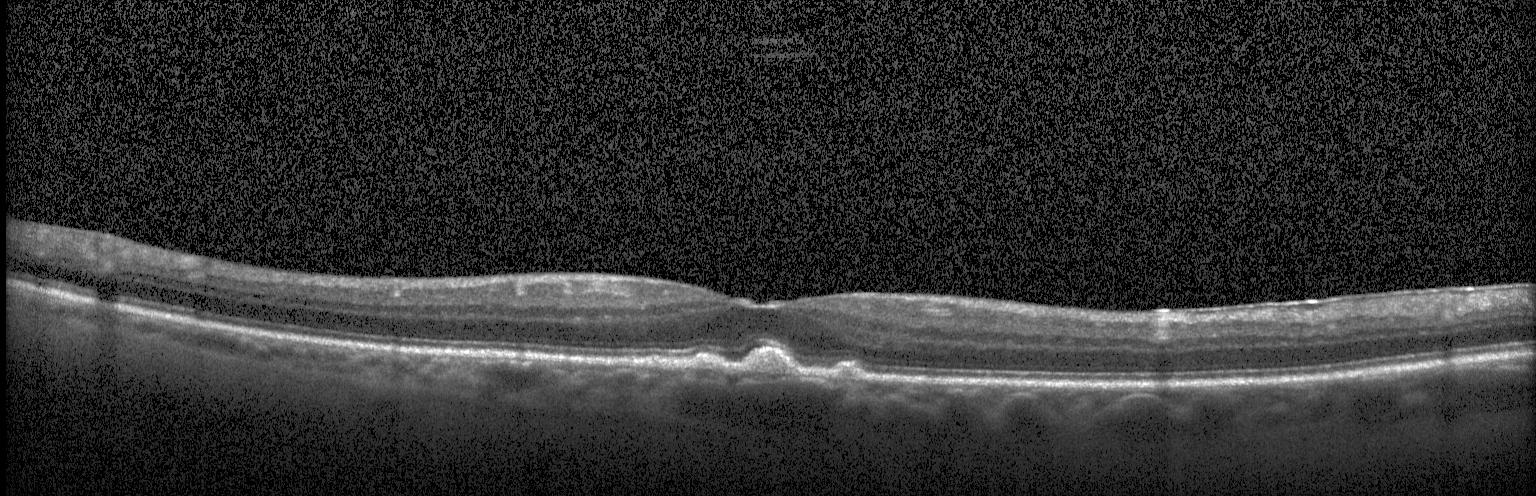
Heidelberg Spectralis OCT system; retinal OCT cross-section. Finding: drusen.